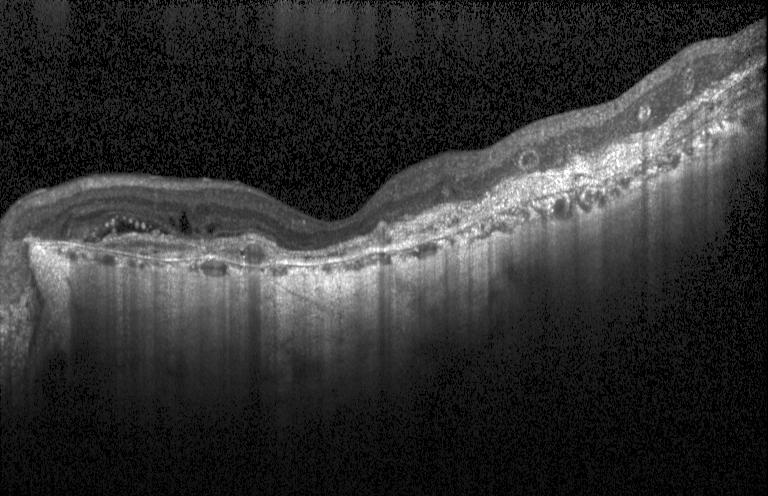 Diagnosis: choroidal neovascularization (CNV).